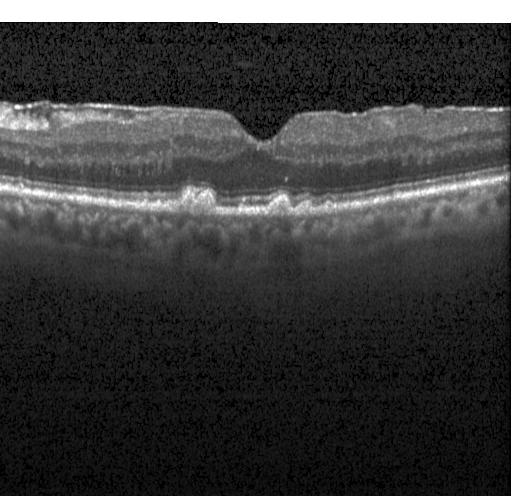

Spectral-domain optical coherence tomography, macular scan, retinal OCT cross-section, acquired on a Heidelberg Spectralis
The scan shows drusen.